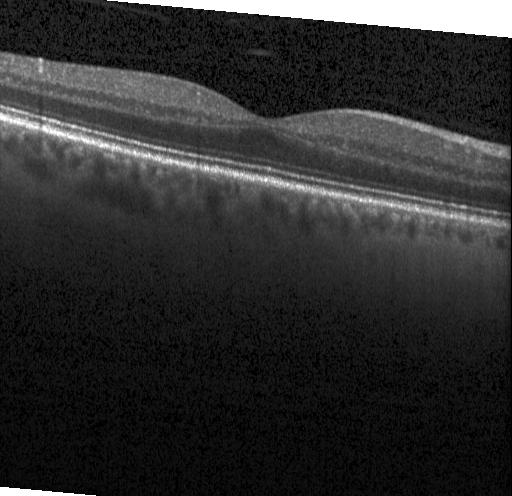

Finding: no evidence of choroidal neovascularization, diabetic macular edema, or drusen.